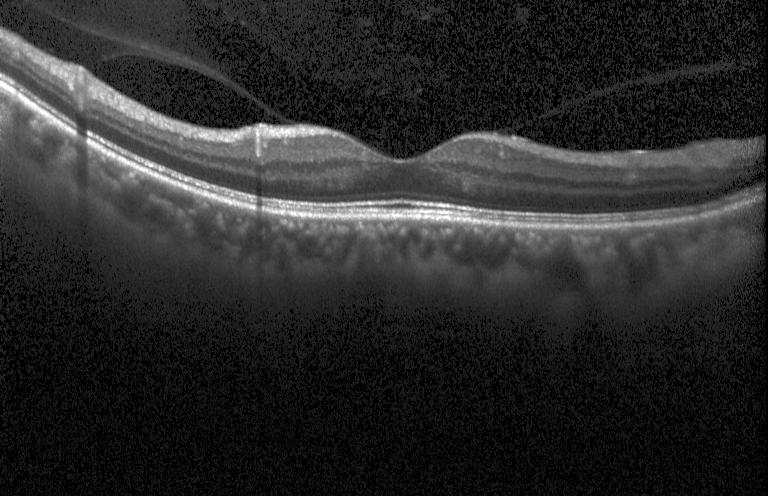

Through the macula, acquired on a Heidelberg Spectralis, retinal OCT B-scan, spectral-domain OCT.
Impression: no CNV, DME, or drusen.